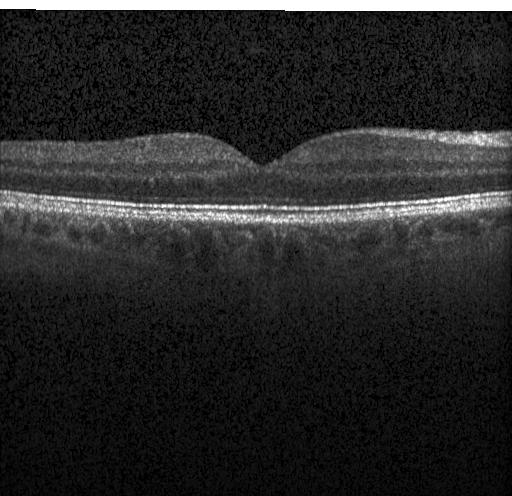 Retinal OCT cross-section; Heidelberg Spectralis OCT system; centered on the fovea
Finding: neither choroidal neovascularization, diabetic macular edema, nor drusen.